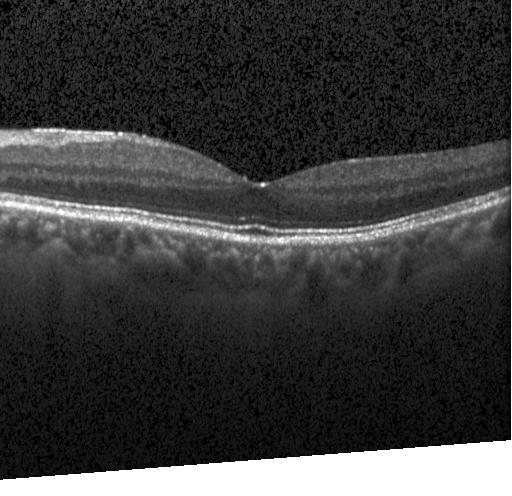

Dx: no choroidal neovascularization, no diabetic macular edema, and no drusen.